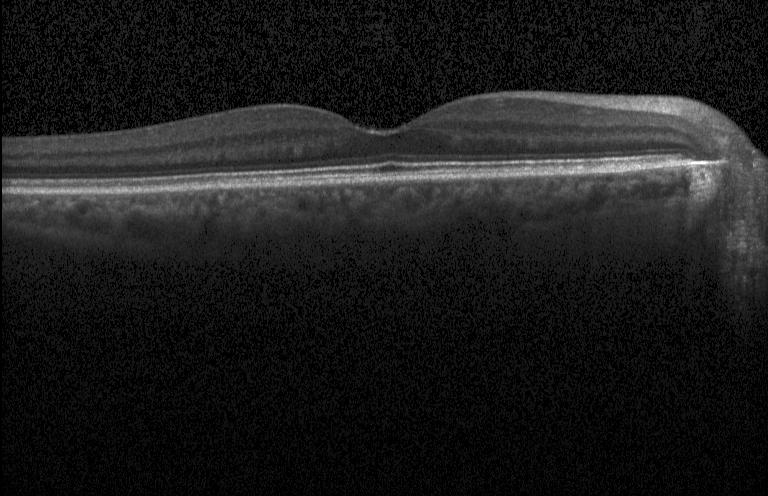 Through the macula; spectral-domain optical coherence tomography; Heidelberg Spectralis; optical coherence tomography scan
Dx: neither choroidal neovascularization, diabetic macular edema, nor drusen.